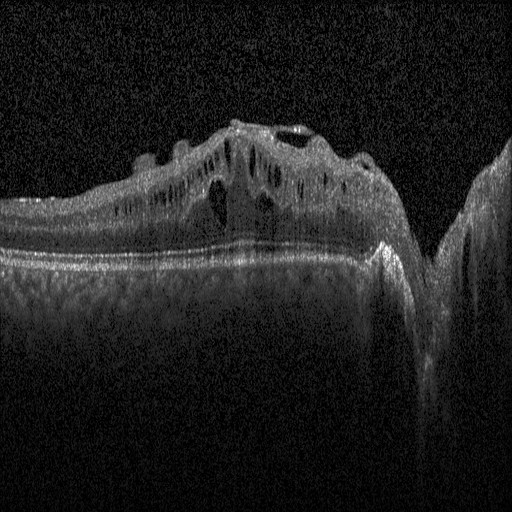
Spectral-domain OCT · retinal OCT cross-section · through the macula · instrument: Heidelberg Spectralis.
Impression: DME.